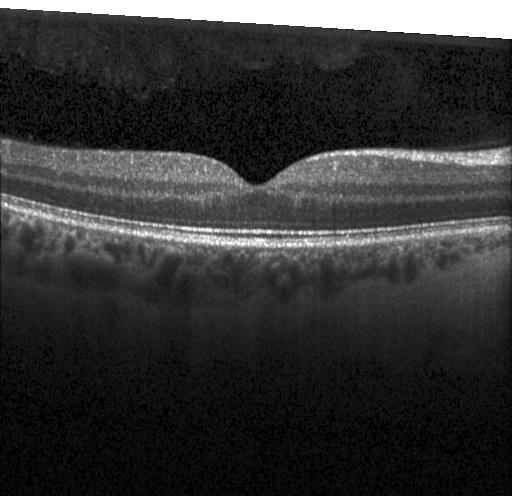

Through the macula. Spectral-domain OCT. Retinal OCT cross-section
Diagnosis: no choroidal neovascularization, no diabetic macular edema, and no drusen.